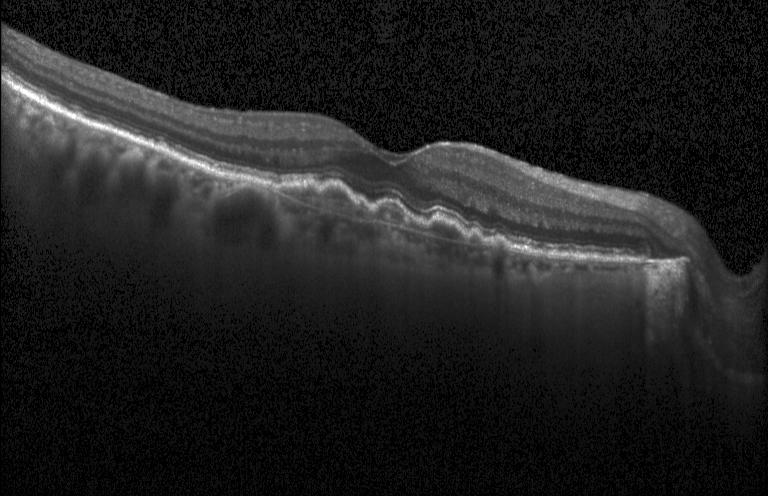

Diagnosis: a choroidal neovascular membrane.